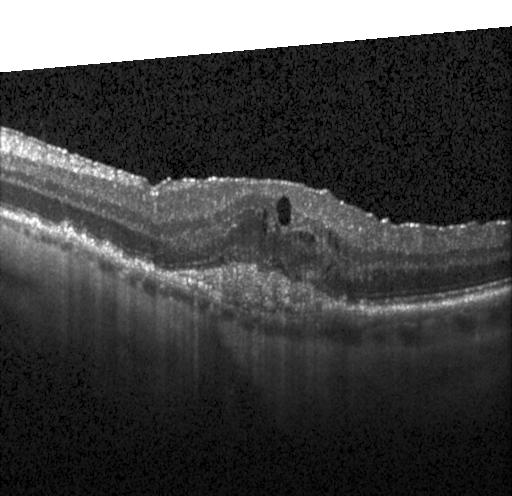
The scan shows a choroidal neovascular membrane.